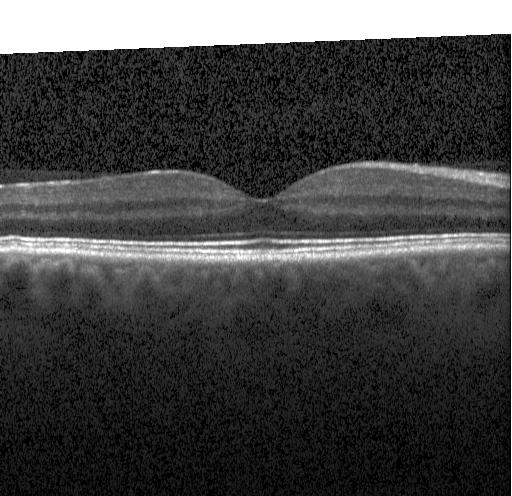

SD-OCT, OCT line scan. Impression: no choroidal neovascularization, diabetic macular edema, or drusen.